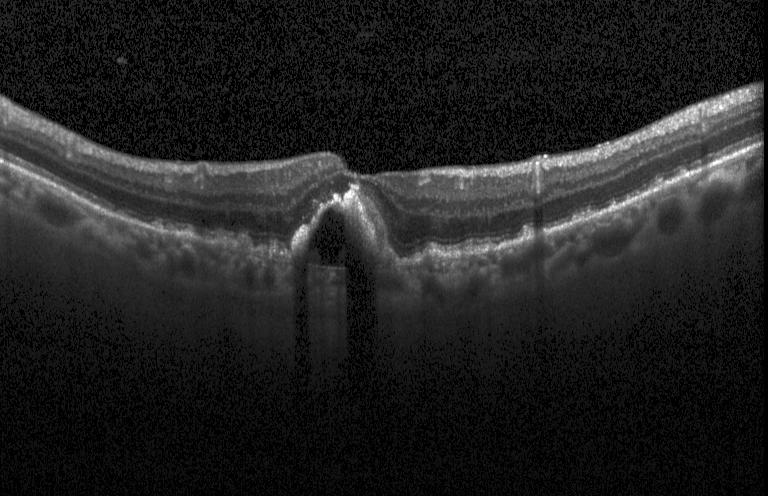
This B-scan demonstrates CNV.